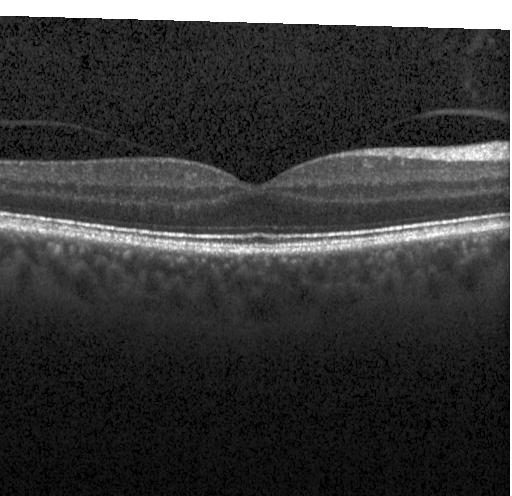 Dx: neither choroidal neovascularization, diabetic macular edema, nor drusen.